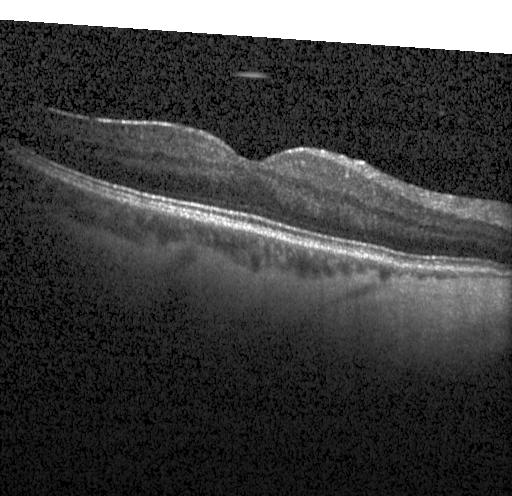

Diagnosis: no CNV, DME, or drusen.